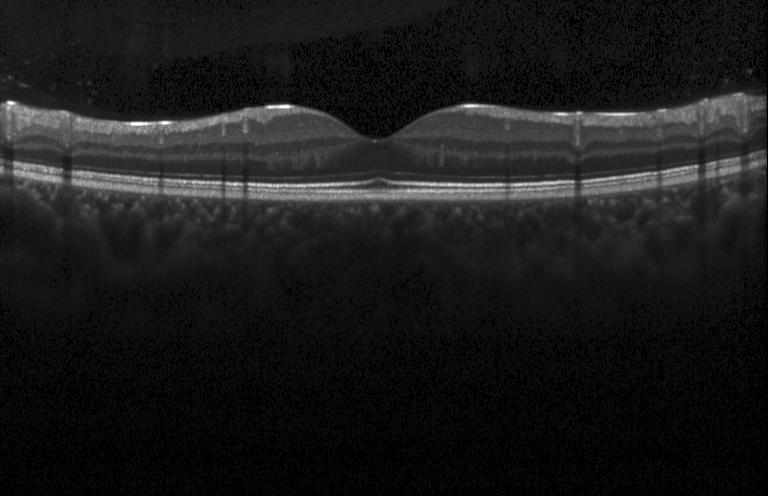
Assessment: neither CNV, DME, nor drusen.